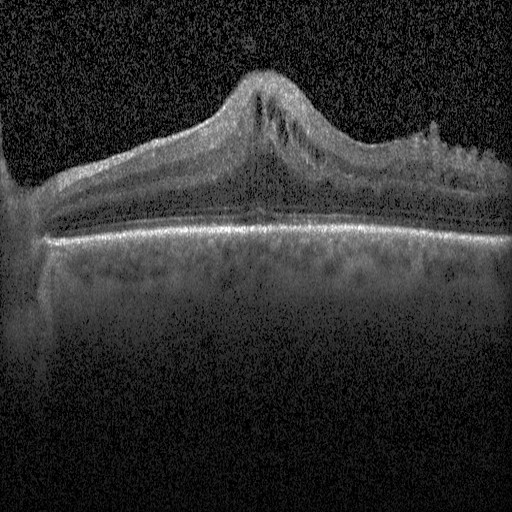

Diagnosis: diabetic macular edema (DME).